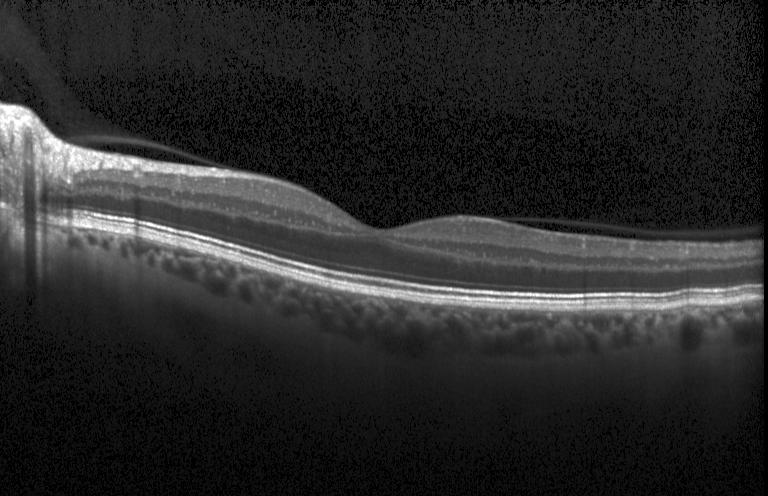

The scan shows no choroidal neovascularization, diabetic macular edema, or drusen.